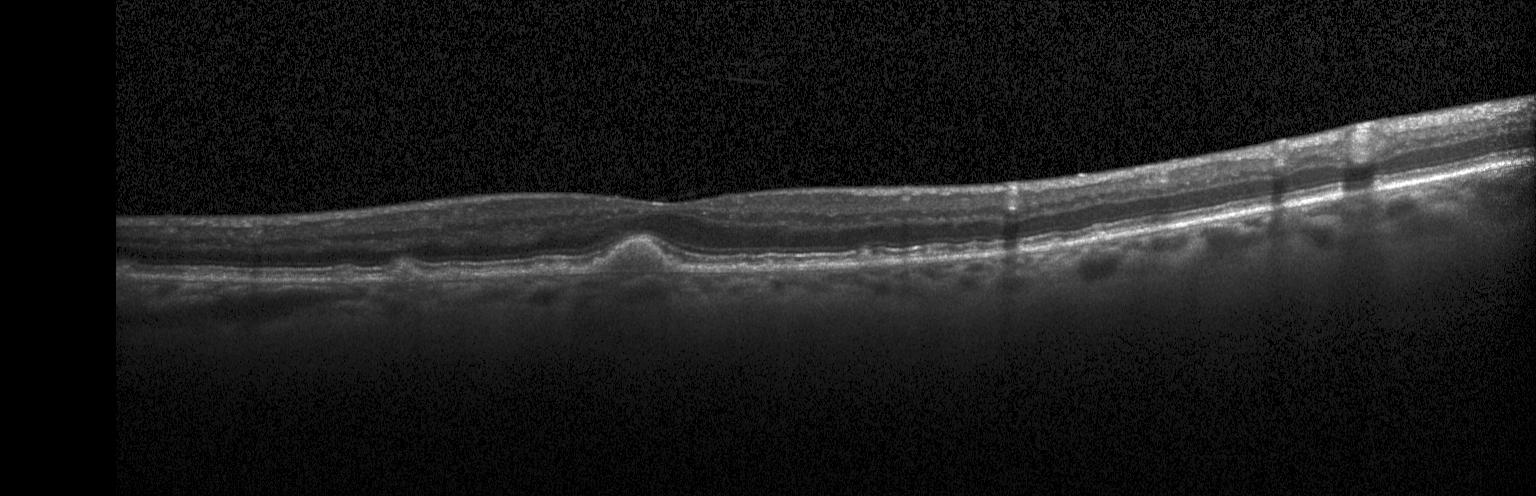
The scan shows drusen.